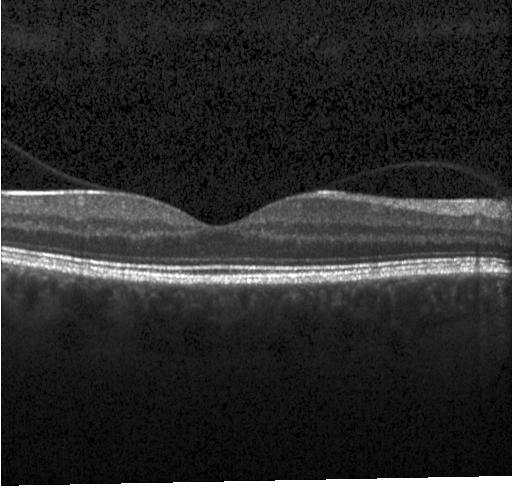 Spectral-domain OCT · OCT B-scan · centered on the fovea · Heidelberg Spectralis OCT system.
Macular OCT: neither choroidal neovascularization, diabetic macular edema, nor drusen.